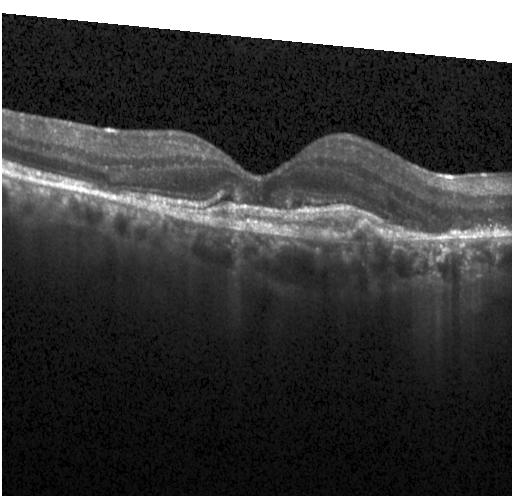
Macular OCT demonstrating CNV.